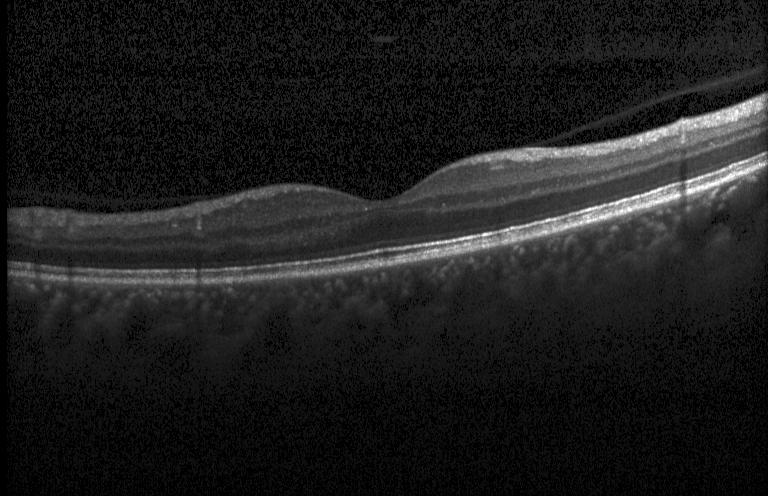
Macular OCT: no CNV, no DME, and no drusen.